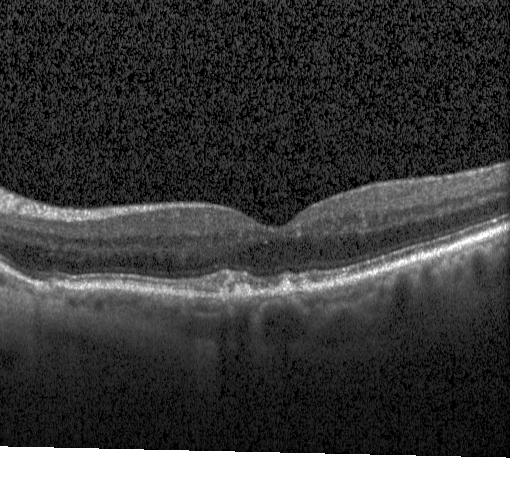

Spectral-domain OCT; retinal OCT B-scan; Heidelberg Spectralis OCT system
Macular OCT: multiple drusen.